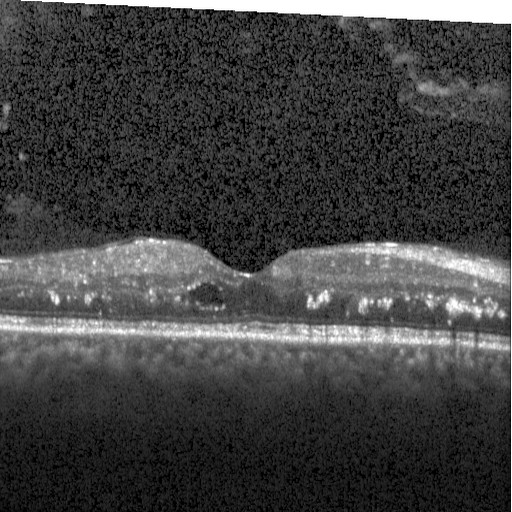
Diagnosis: diabetic macular edema (DME).